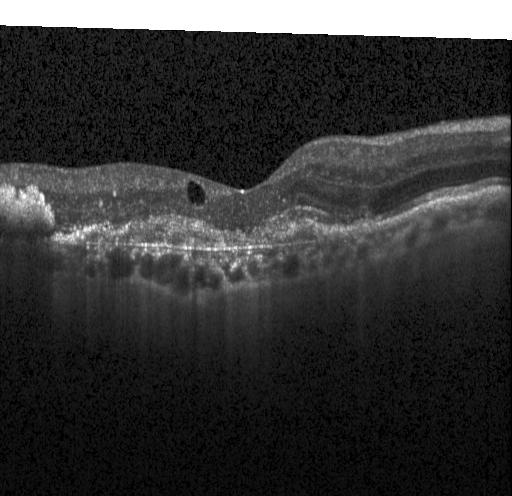
OCT line scan; macular scan. Macular OCT: CNV.